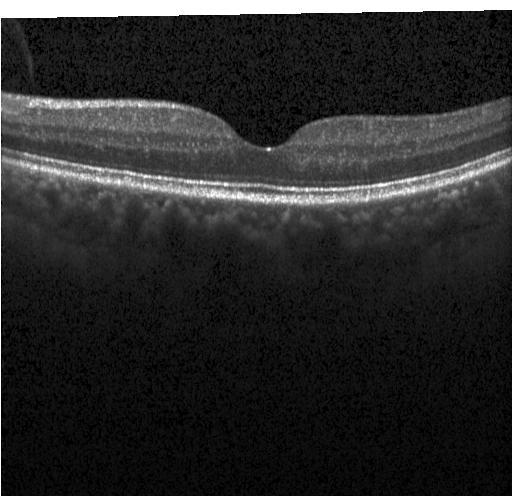
Instrument: Heidelberg Spectralis. Optical coherence tomography B-scan.
Finding: no evidence of CNV, DME, or drusen.